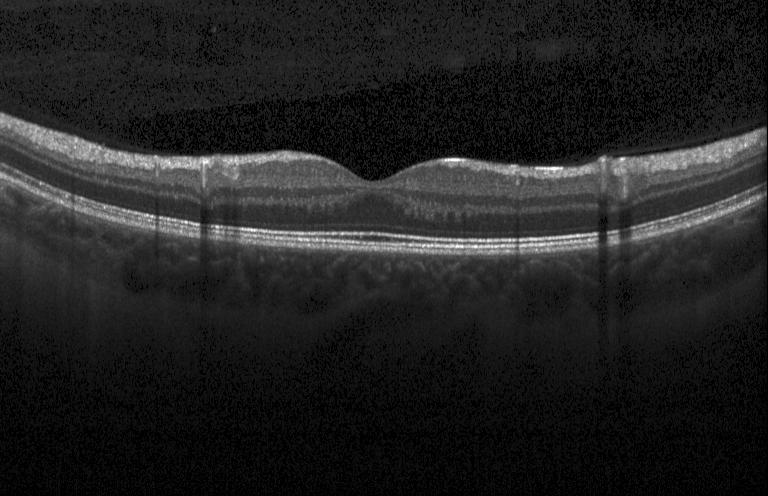

Macular scan, retinal OCT B-scan
Finding: no choroidal neovascularization, diabetic macular edema, or drusen.